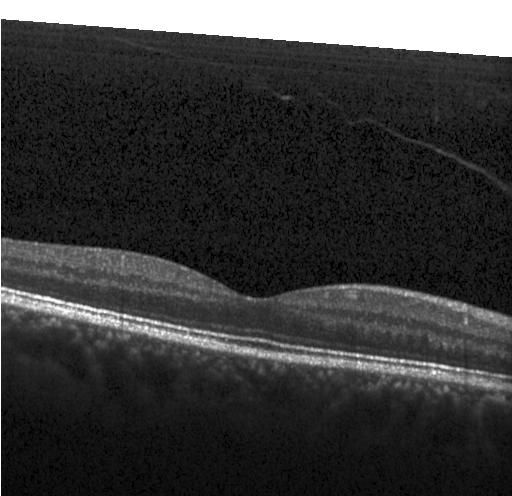 Impression: no CNV, no DME, and no drusen.